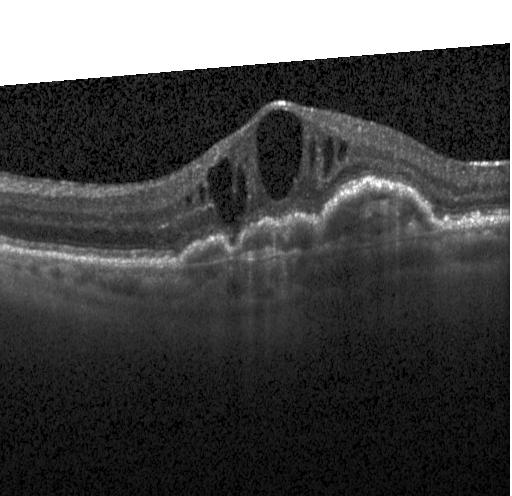
OCT line scan. Finding: CNV.